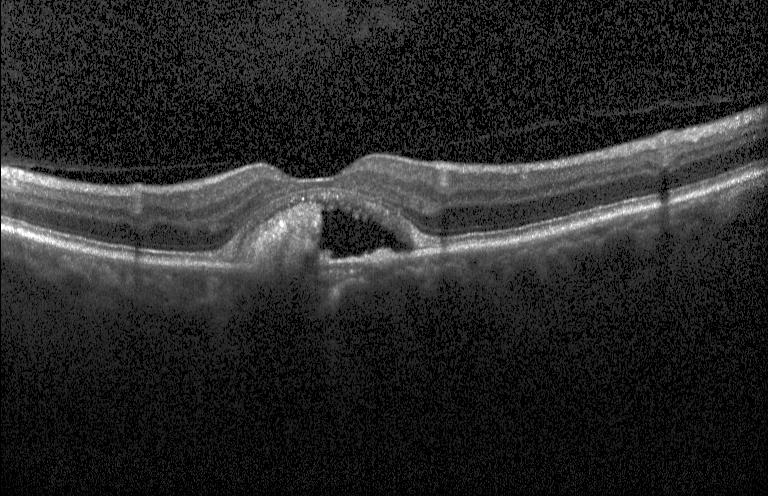 OCT scan showing choroidal neovascularization.